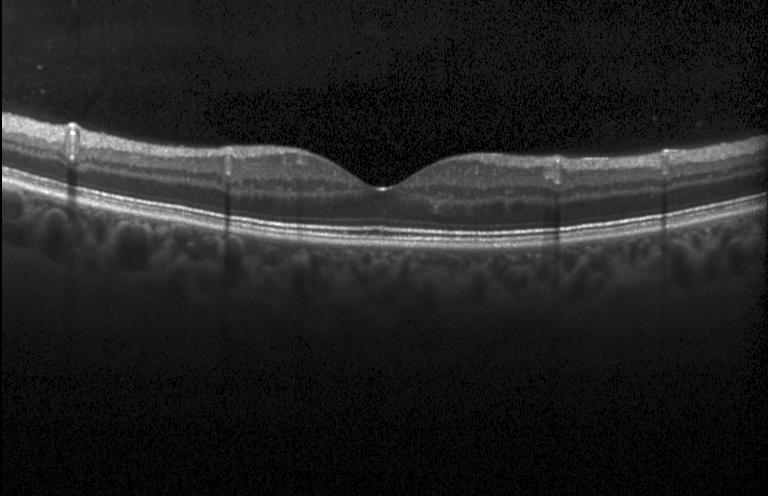 Optical coherence tomography B-scan · instrument: Heidelberg Spectralis
This B-scan demonstrates no evidence of CNV, DME, or drusen.